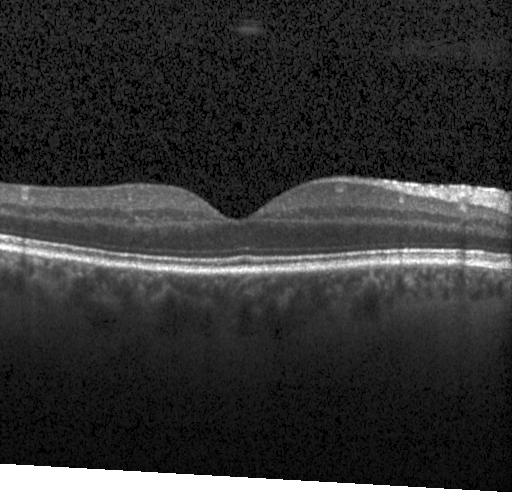 The scan shows no evidence of CNV, DME, or drusen.